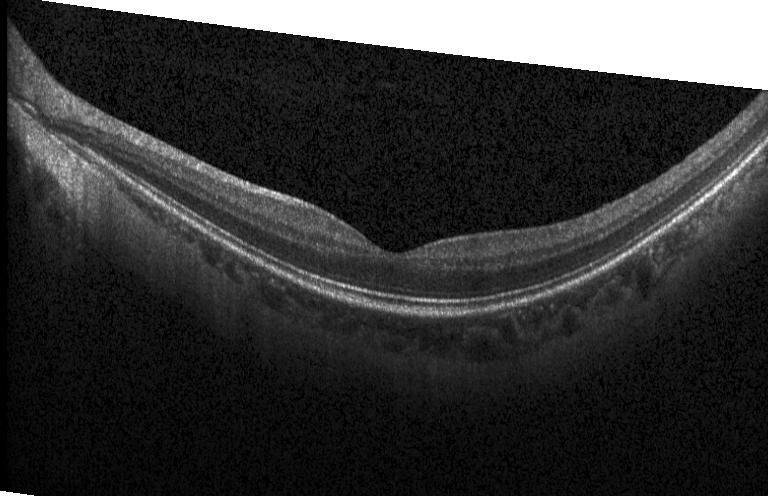

Optical coherence tomography B-scan — Finding: neither CNV, DME, nor drusen.